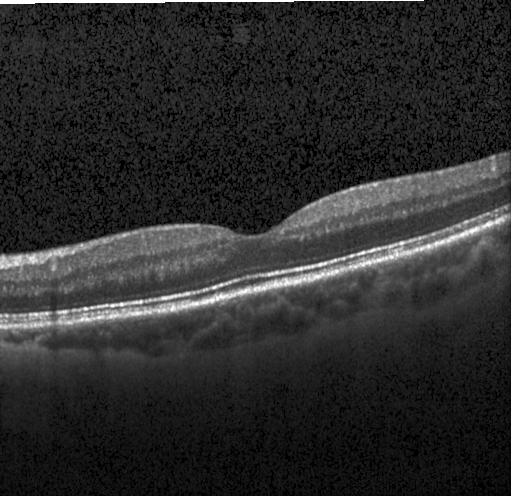

Instrument: Heidelberg Spectralis. Spectral-domain OCT. Centered on the fovea. OCT line scan — Finding: neither choroidal neovascularization, diabetic macular edema, nor drusen.